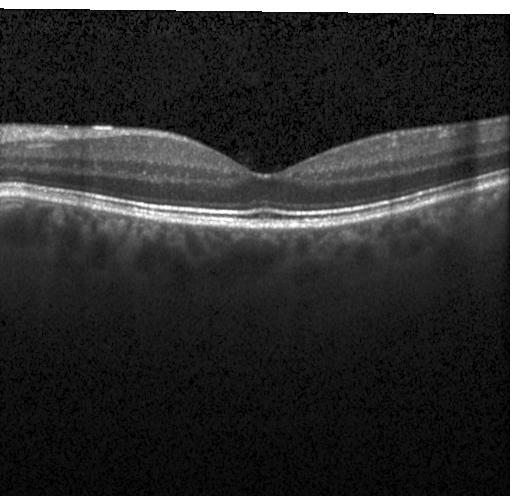

Macular OCT: no CNV, no DME, and no drusen.